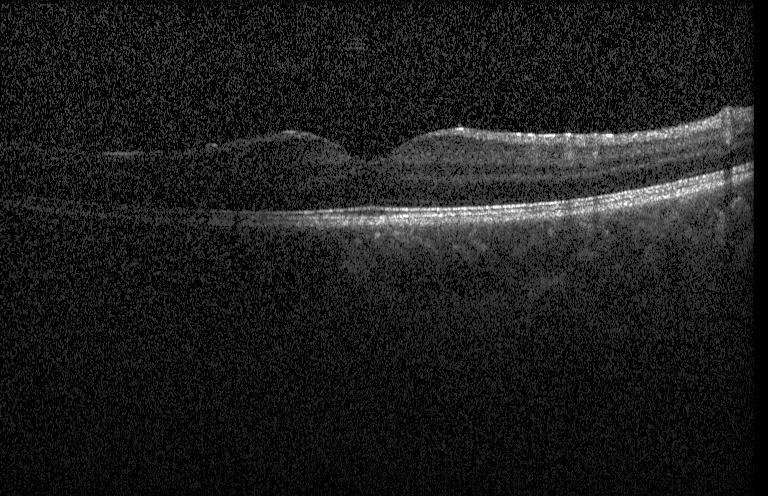 Spectral-domain optical coherence tomography · through the macula · optical coherence tomography scan. Impression: no choroidal neovascularization, no diabetic macular edema, and no drusen.